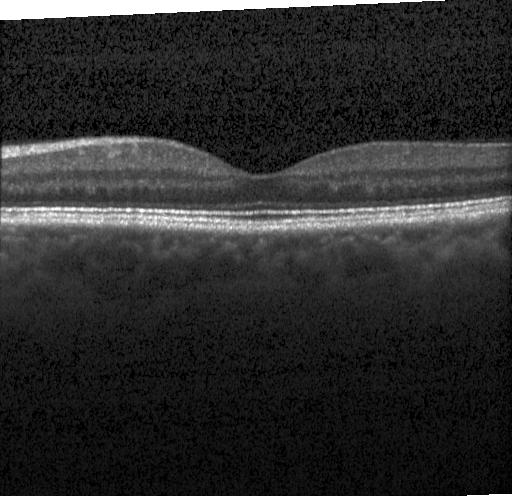
Finding: no evidence of choroidal neovascularization, diabetic macular edema, or drusen.